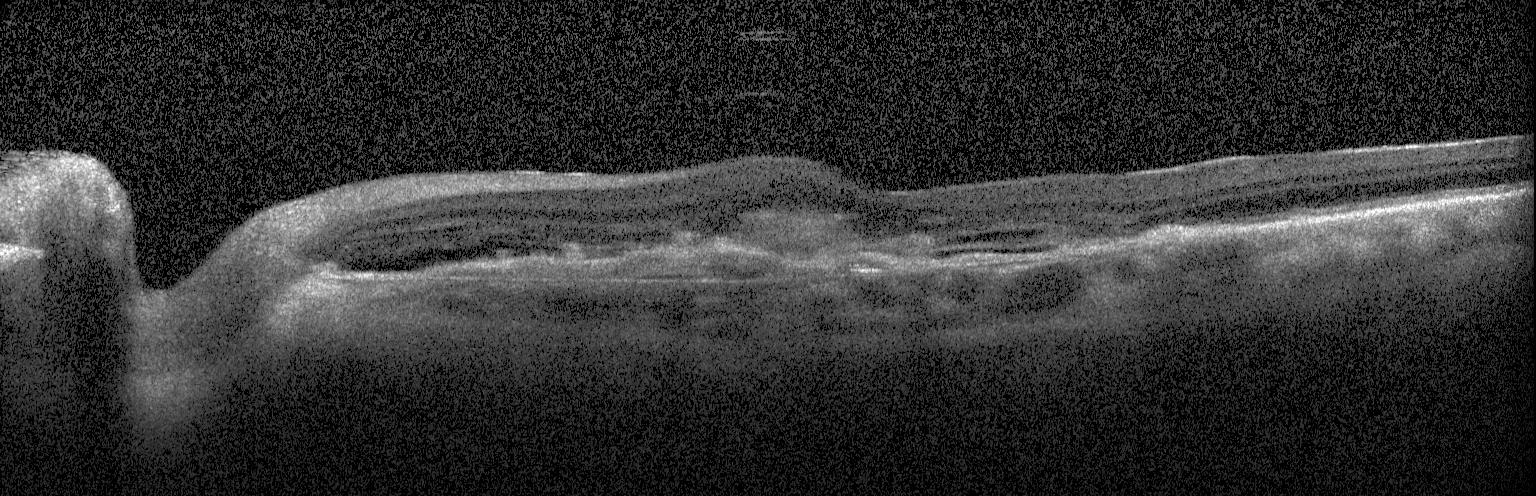
Fovea-centered, optical coherence tomography scan.
Dx: choroidal neovascularization (CNV).